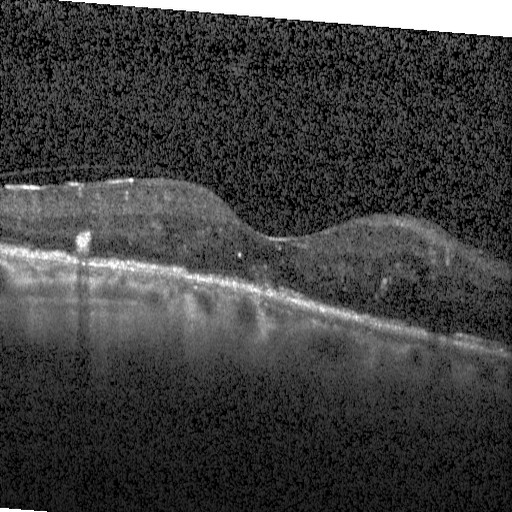

Impression: DME.